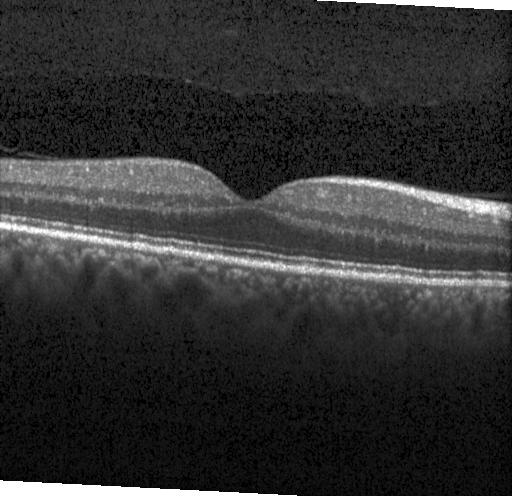

Spectral-domain OCT. Macular scan. Heidelberg Spectralis OCT system. OCT line scan — Impression: no choroidal neovascularization, diabetic macular edema, or drusen.